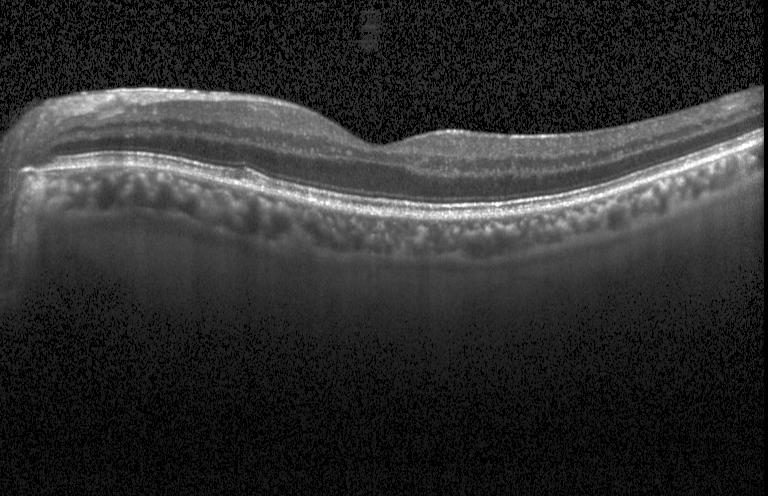 Optical coherence tomography scan, SD-OCT. Drusen.